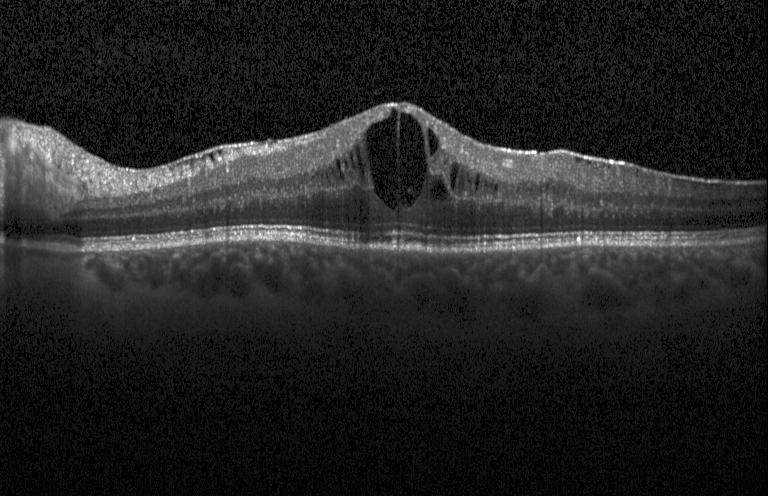 Macular scan, optical coherence tomography scan, SD-OCT — Assessment: diabetic macular edema.